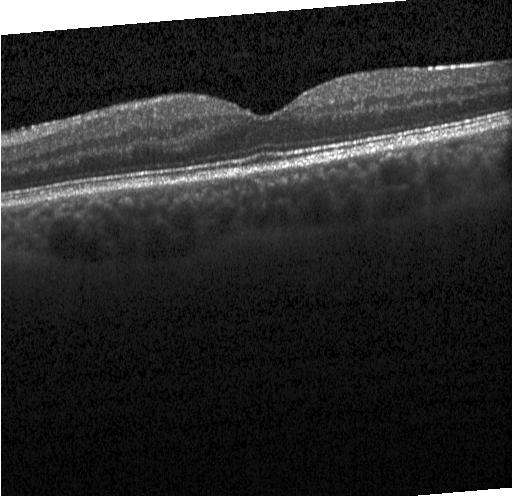 Assessment: no choroidal neovascularization, no diabetic macular edema, and no drusen.